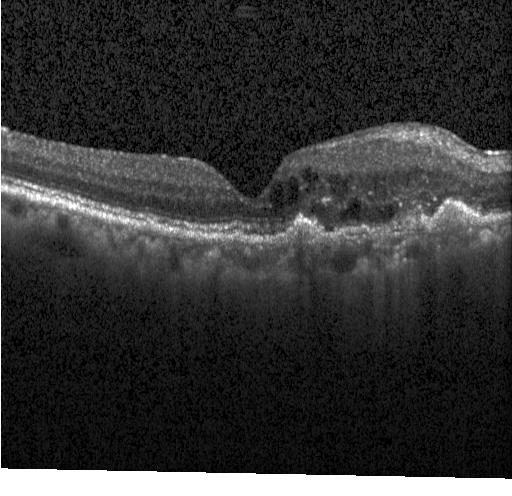
Spectral-domain optical coherence tomography, retinal OCT cross-section, macular scan, instrument: Heidelberg Spectralis — Diagnosis: choroidal neovascularization.